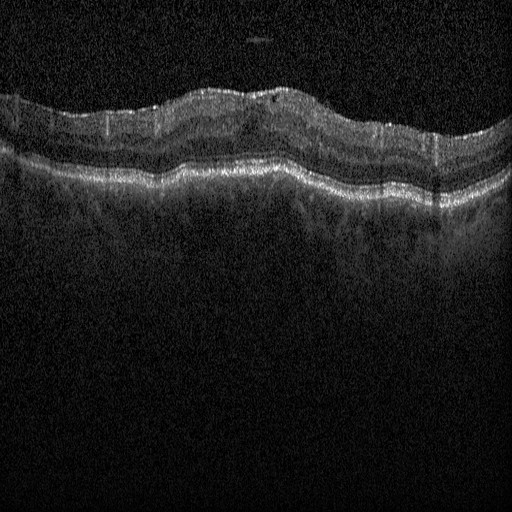
Centered on the fovea · Heidelberg Spectralis OCT system · SD-OCT · retinal OCT B-scan.
OCT finding: diabetic macular edema.